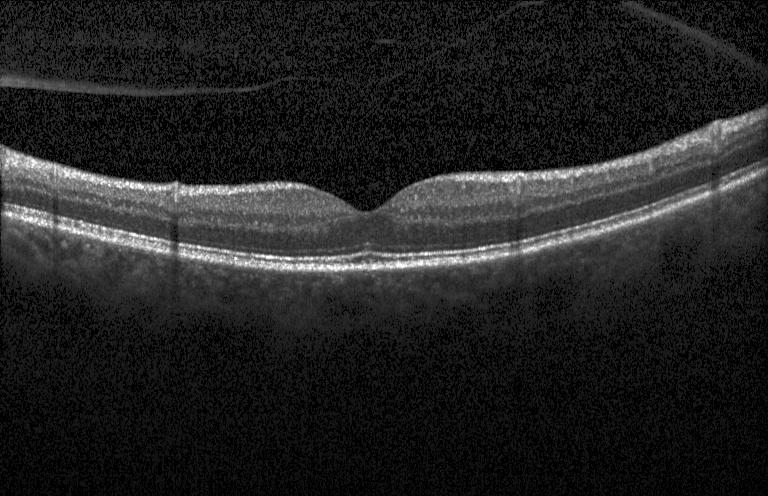

Spectral-domain OCT. Optical coherence tomography scan. Acquired on a Heidelberg Spectralis.
The scan shows no choroidal neovascularization, no diabetic macular edema, and no drusen.